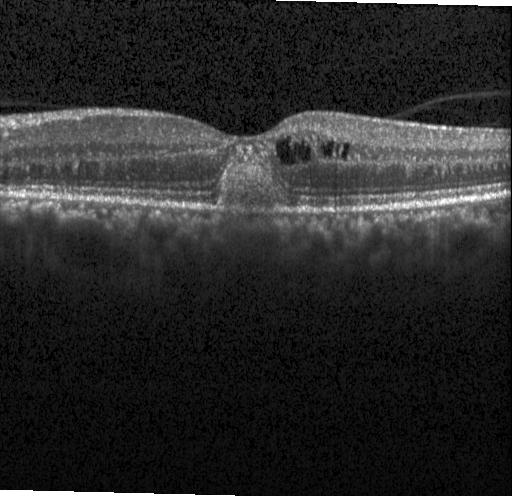
Impression: choroidal neovascularization.